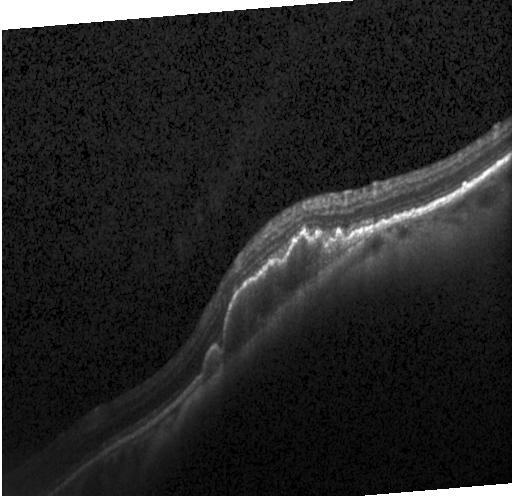 Macular scan. Spectral-domain optical coherence tomography. Retinal OCT B-scan. Instrument: Heidelberg Spectralis.
Dx: choroidal neovascularization.